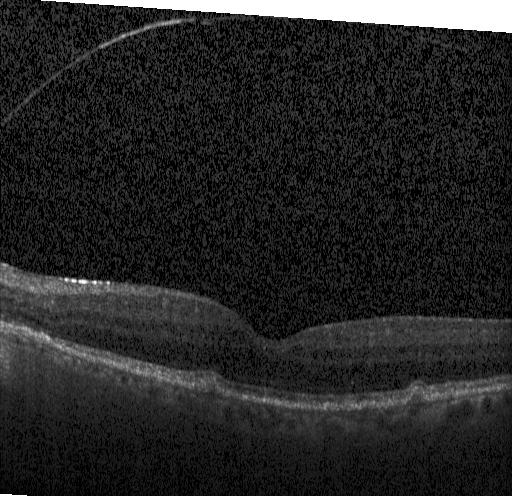 Macular OCT demonstrating sub-RPE drusenoid deposits.